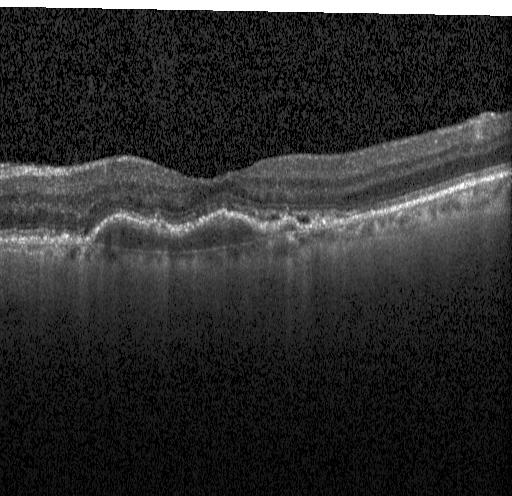 A choroidal neovascular membrane.